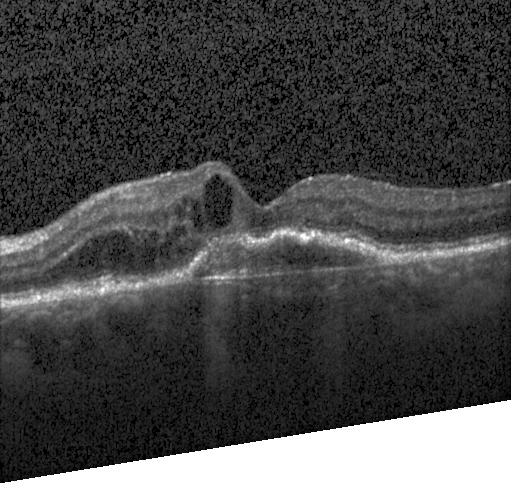

Diagnosis: CNV.